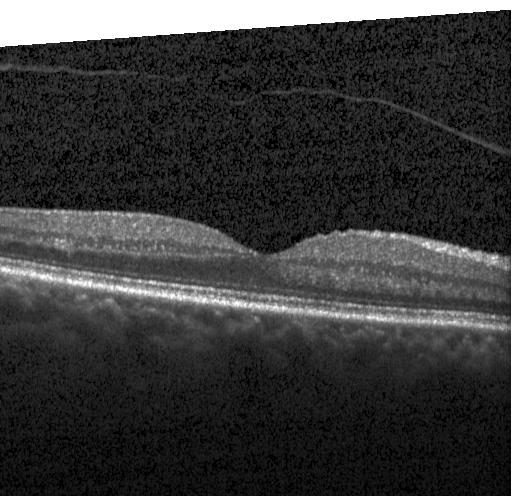 OCT B-scan, instrument: Heidelberg Spectralis, spectral-domain OCT, fovea-centered. Impression: neither CNV, DME, nor drusen.